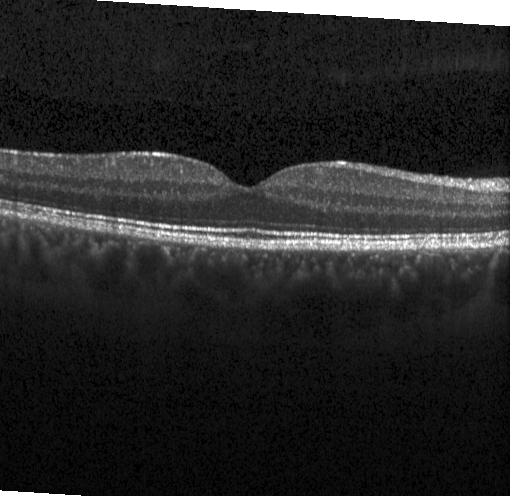 Retinal OCT cross-section, centered on the fovea, spectral-domain optical coherence tomography.
Impression: neither choroidal neovascularization, diabetic macular edema, nor drusen.